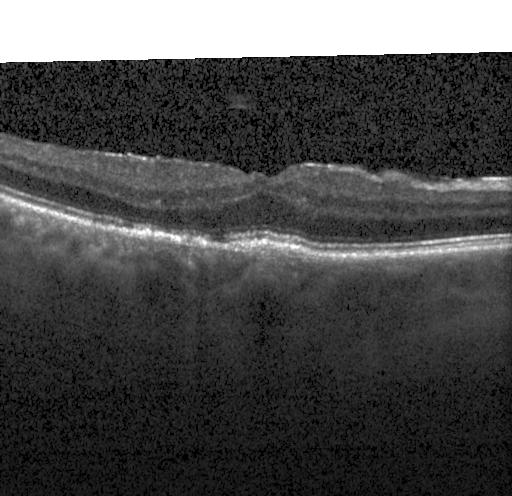

Macular scan, optical coherence tomography scan
Impression: a choroidal neovascular membrane.